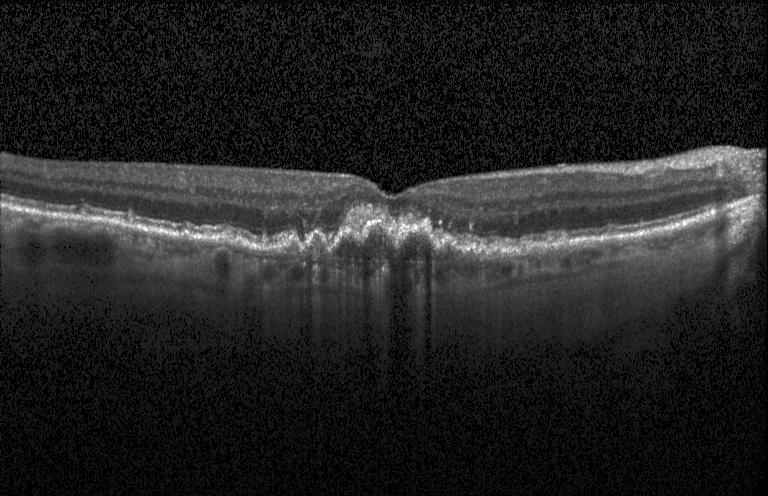

Acquired on a Heidelberg Spectralis · OCT B-scan · SD-OCT. Impression: choroidal neovascularization (CNV).